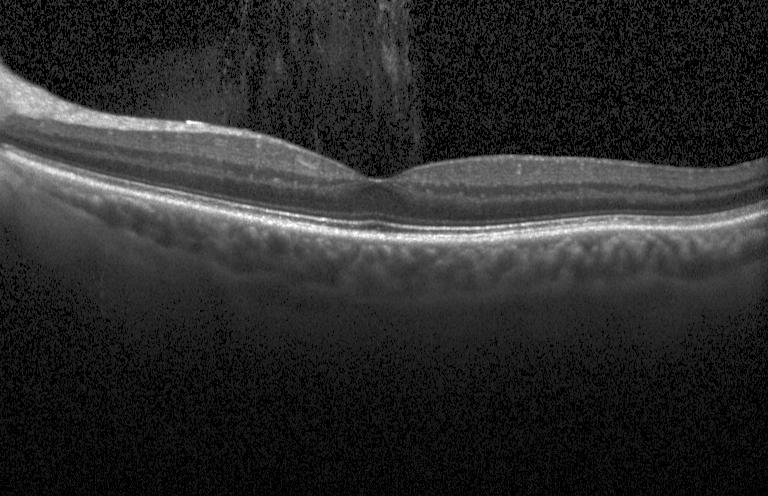 Retinal OCT cross-section.
Finding: neither CNV, DME, nor drusen.